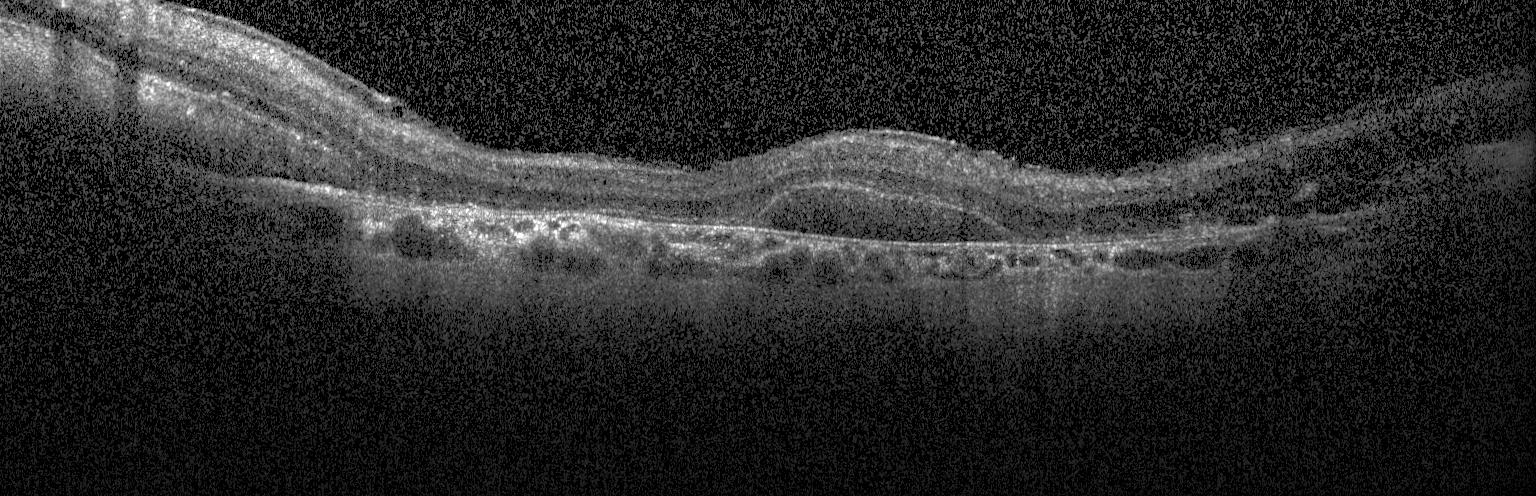

Retinal OCT cross-section
Diagnosis: a choroidal neovascular membrane.